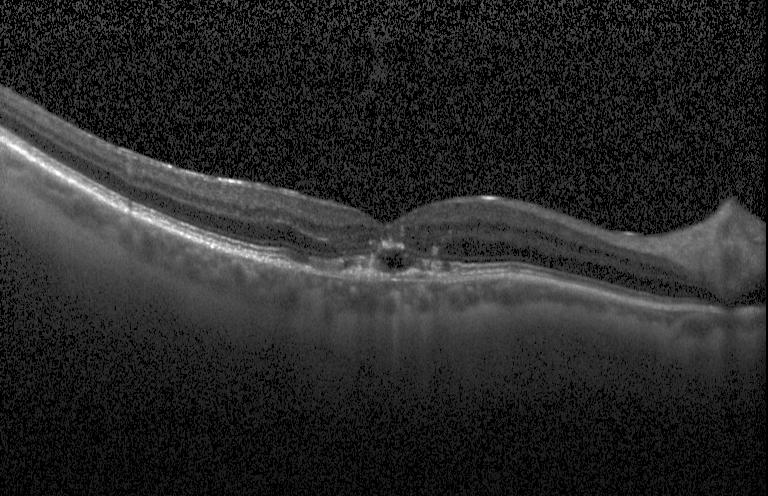

Retinal OCT B-scan · spectral-domain optical coherence tomography
Assessment: CNV.